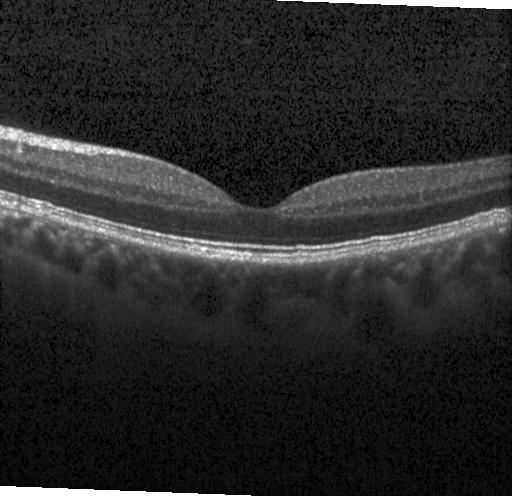
OCT scan showing no choroidal neovascularization, diabetic macular edema, or drusen.